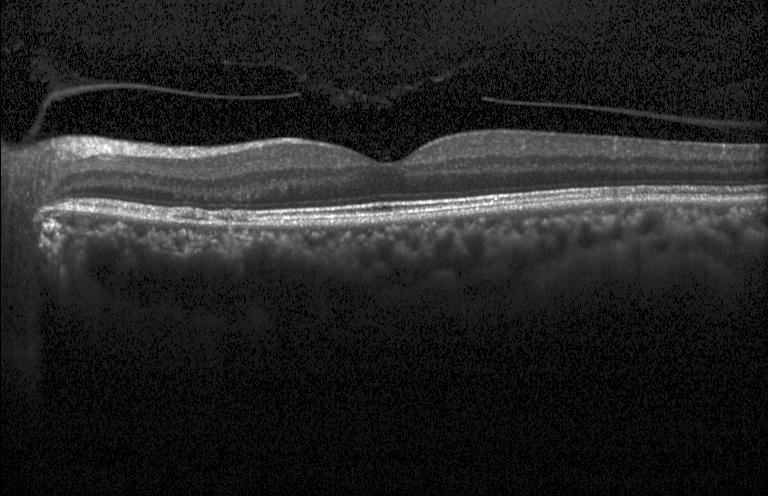
Retinal OCT cross-section, Heidelberg Spectralis OCT system, horizontal scan through the fovea
Impression: neither choroidal neovascularization, diabetic macular edema, nor drusen.